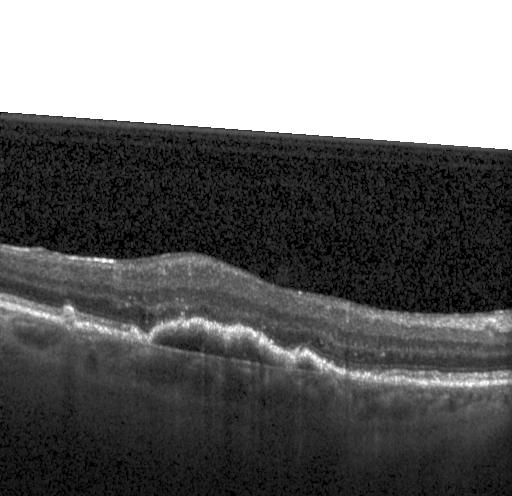

Optical coherence tomography scan, instrument: Heidelberg Spectralis, through the macula — Impression: a choroidal neovascular membrane.